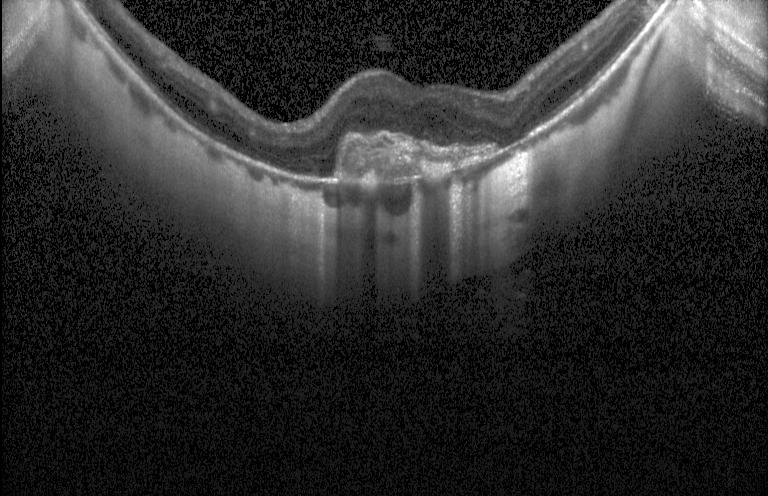 OCT line scan · Heidelberg Spectralis OCT system.
Finding: CNV.